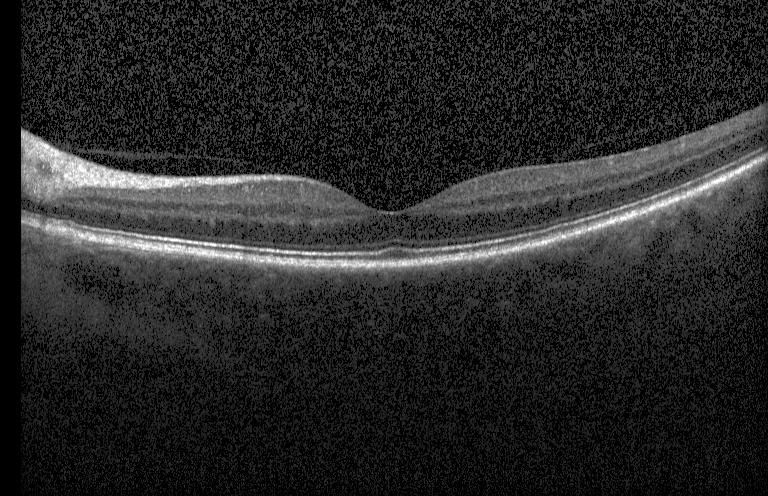 Optical coherence tomography scan. Macular OCT: no CNV, DME, or drusen.